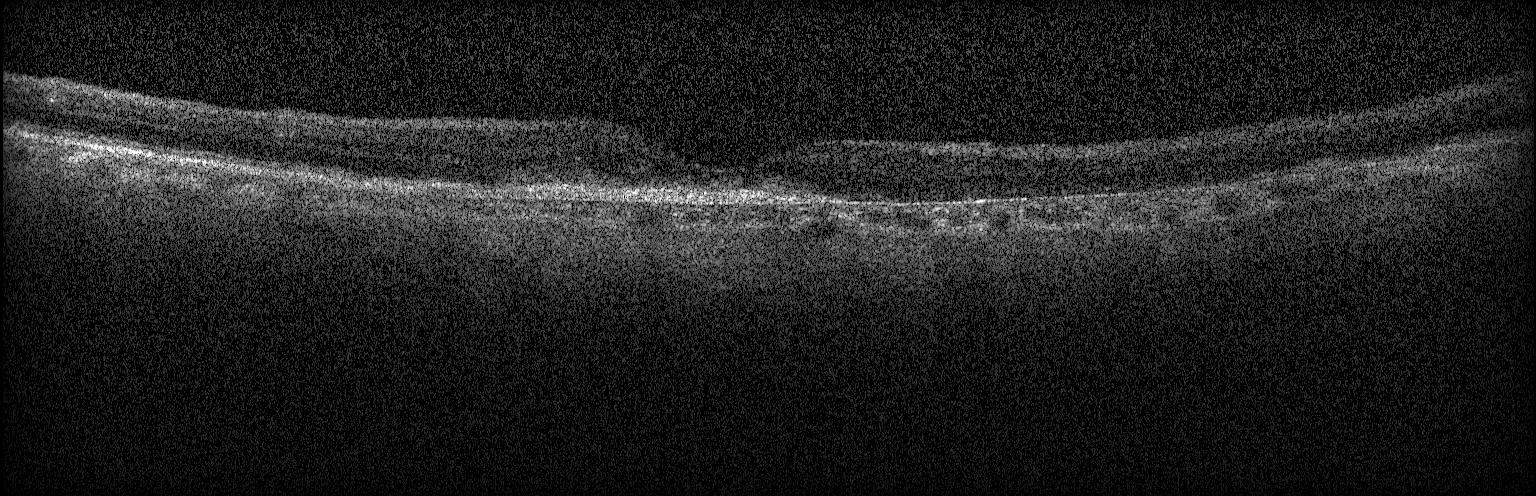
OCT B-scan showing choroidal neovascularization.